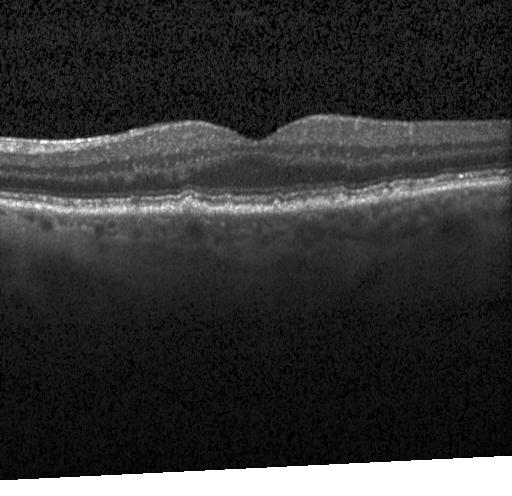
Diagnosis: multiple drusen.